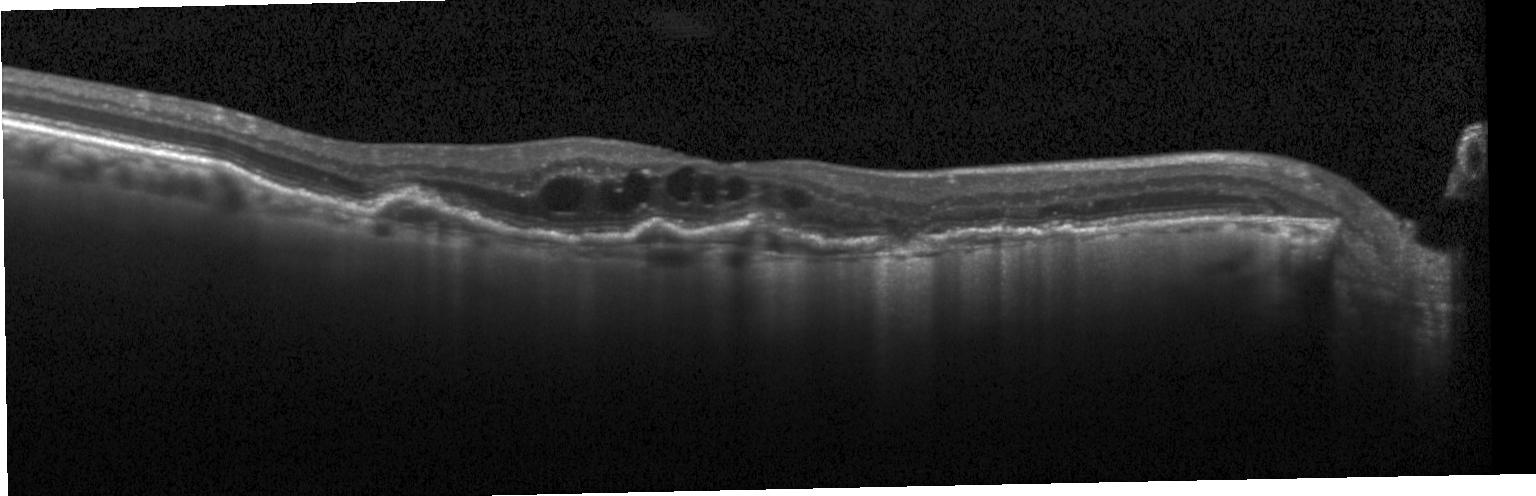

OCT B-scan, through the macula.
Assessment: a choroidal neovascular membrane.